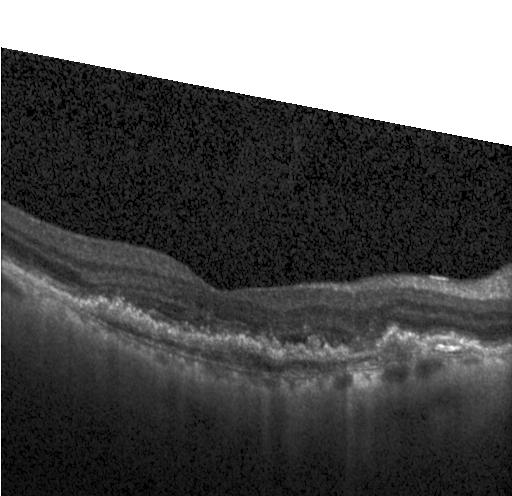 Dx: CNV.